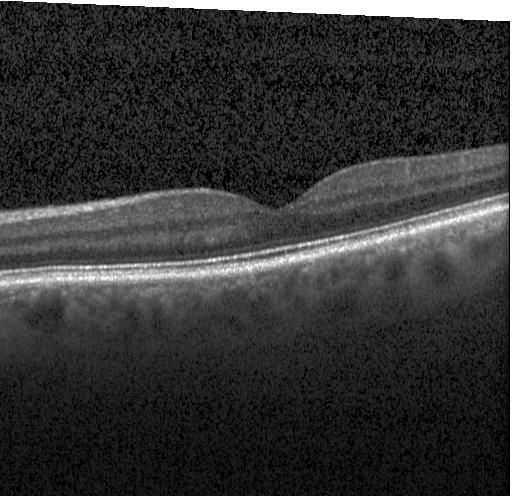
Macular OCT: no evidence of CNV, DME, or drusen.